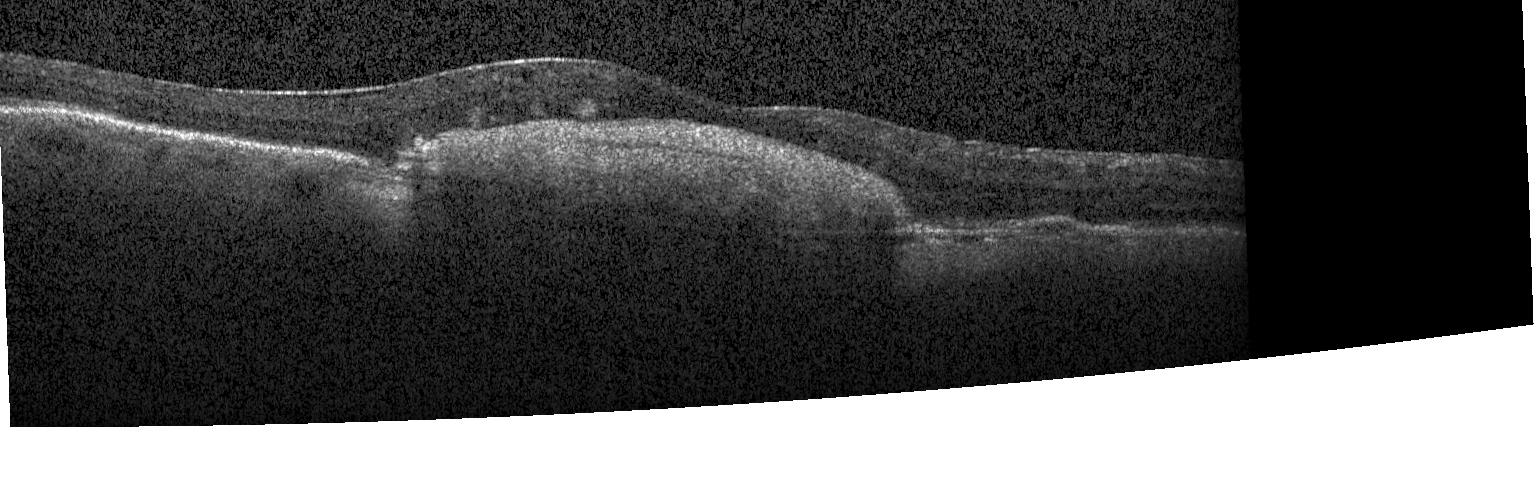
Retinal OCT B-scan, spectral-domain optical coherence tomography, instrument: Heidelberg Spectralis, through the macula. Dx: a choroidal neovascular membrane.